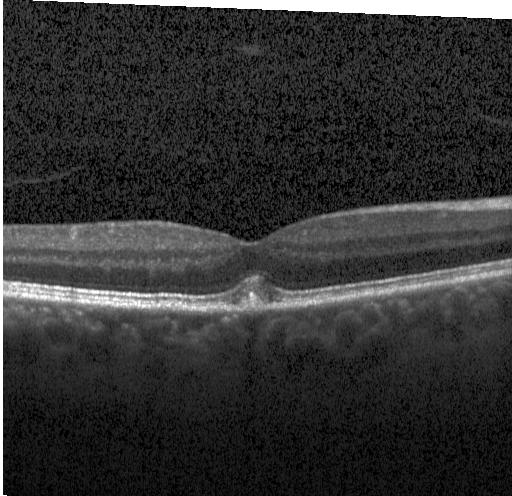

Spectral-domain OCT B-scan: multiple drusen.